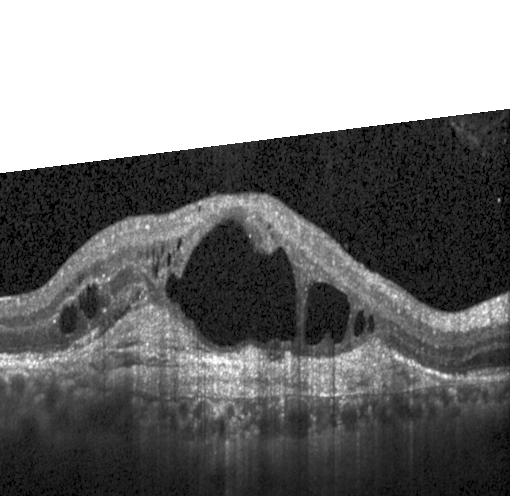 Spectral-domain optical coherence tomography; optical coherence tomography B-scan — This B-scan demonstrates a choroidal neovascular membrane.